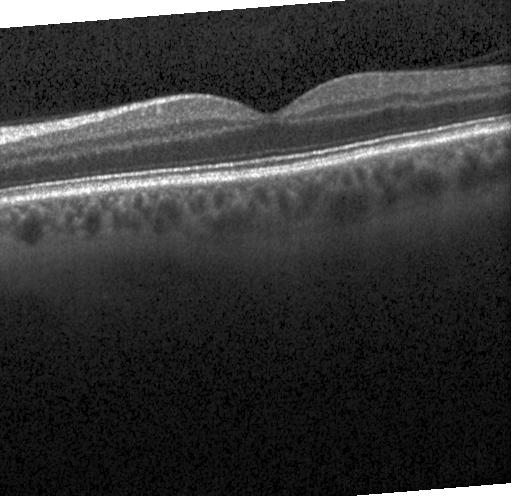

Spectral-domain optical coherence tomography; centered on the fovea; retinal OCT cross-section — Impression: no choroidal neovascularization, no diabetic macular edema, and no drusen.